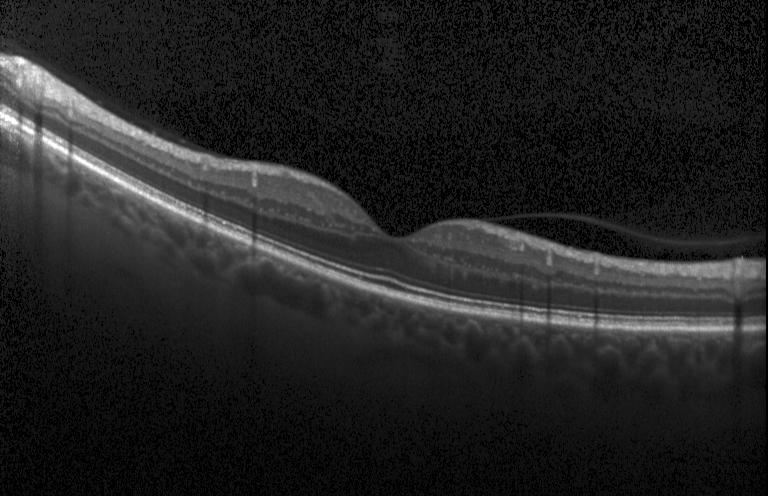 Acquired on a Heidelberg Spectralis; OCT line scan; through the macula; spectral-domain OCT
Neither choroidal neovascularization, diabetic macular edema, nor drusen.